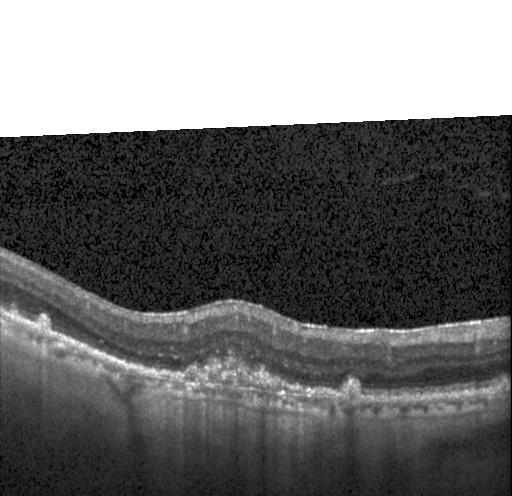

Impression: choroidal neovascularization (CNV).